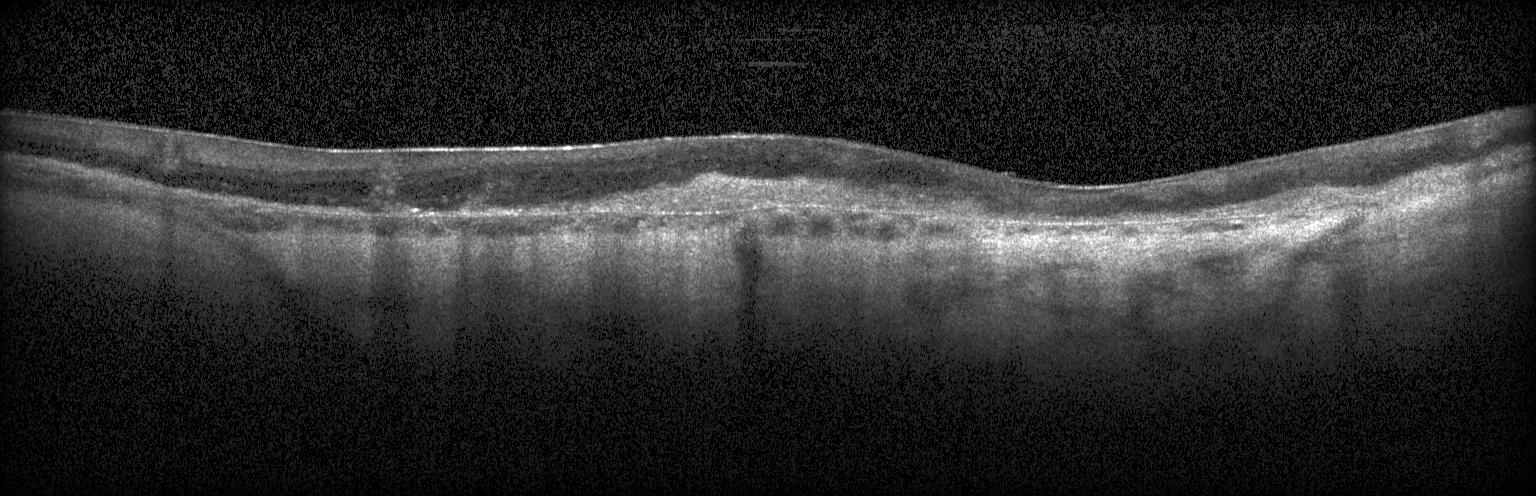 OCT scan showing choroidal neovascularization (CNV).